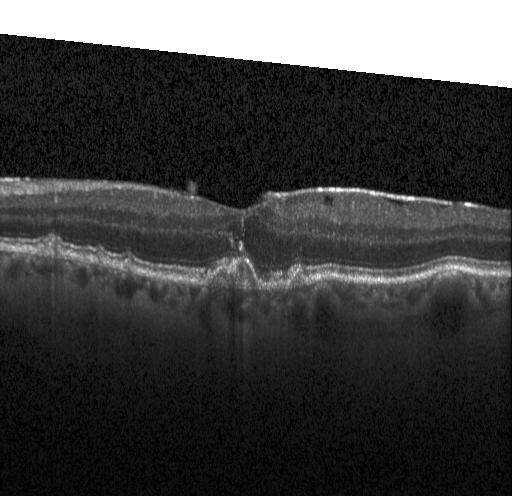
Impression: multiple drusen.